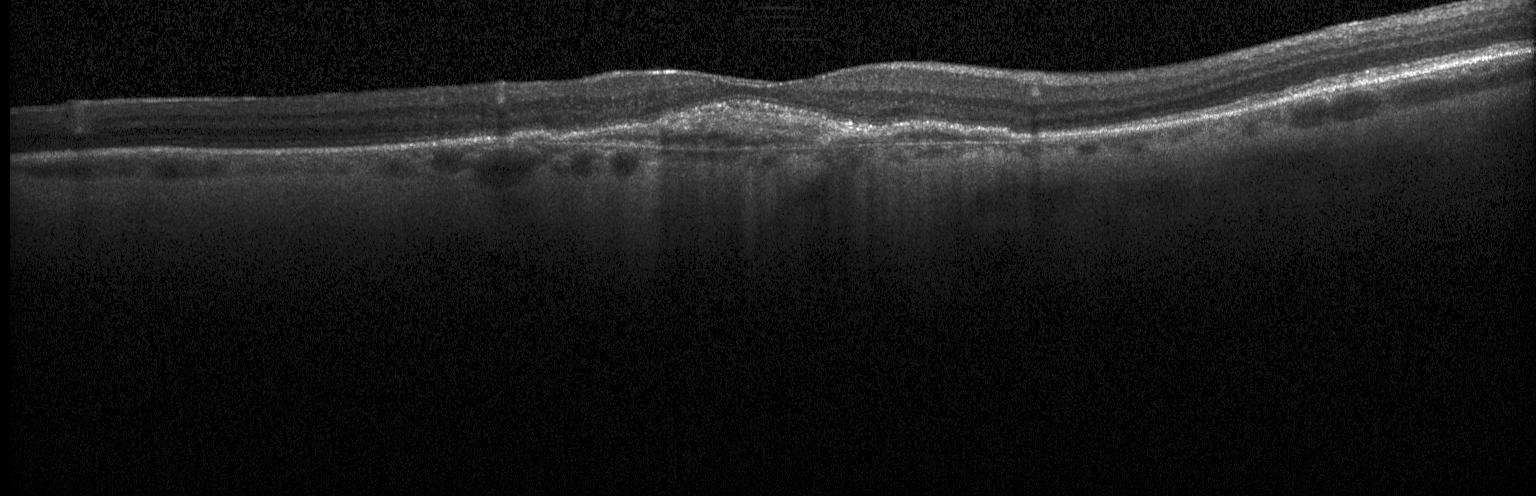 Macular scan. Optical coherence tomography B-scan.
Dx: a choroidal neovascular membrane.